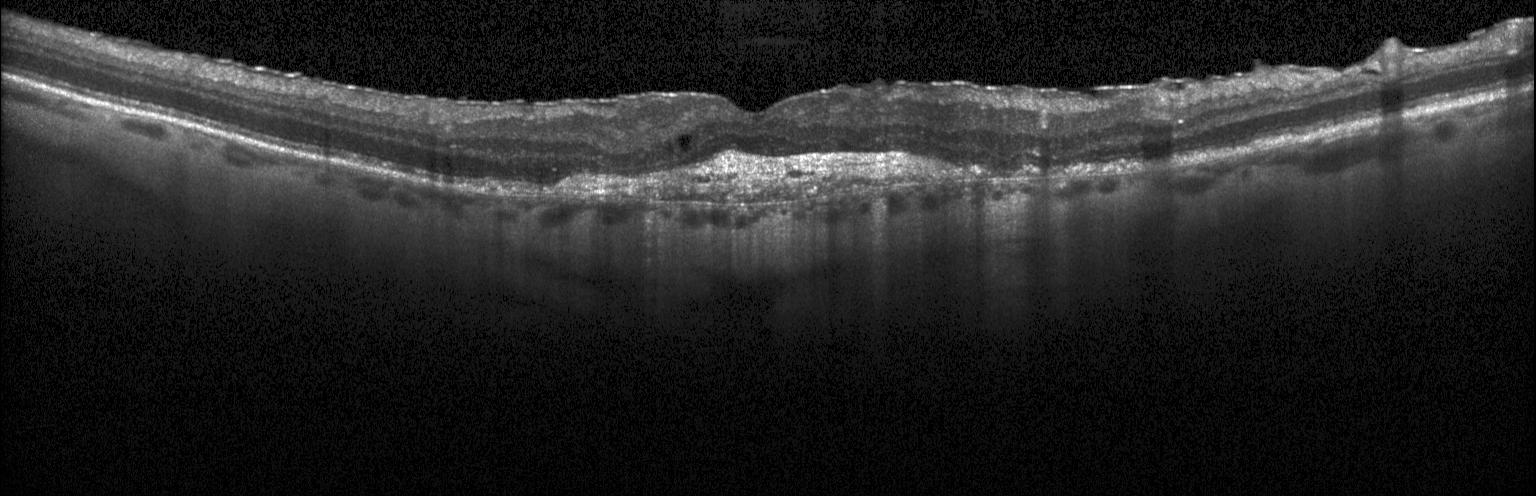

Retinal OCT B-scan; through the macula; SD-OCT.
Assessment: a choroidal neovascular membrane.